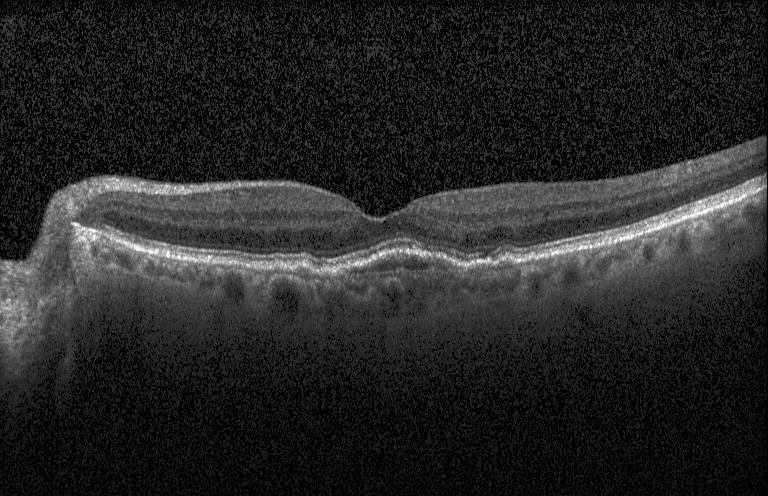 OCT line scan · fovea-centered
This B-scan demonstrates CNV.